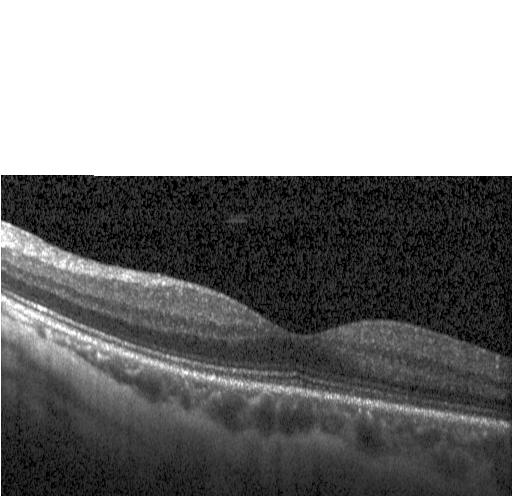 Optical coherence tomography scan.
Impression: no choroidal neovascularization, diabetic macular edema, or drusen.